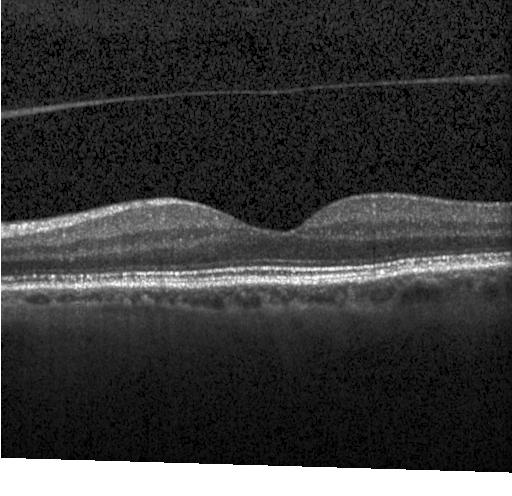
Heidelberg Spectralis OCT system, optical coherence tomography scan, spectral-domain optical coherence tomography, through the macula. OCT finding: neither CNV, DME, nor drusen.